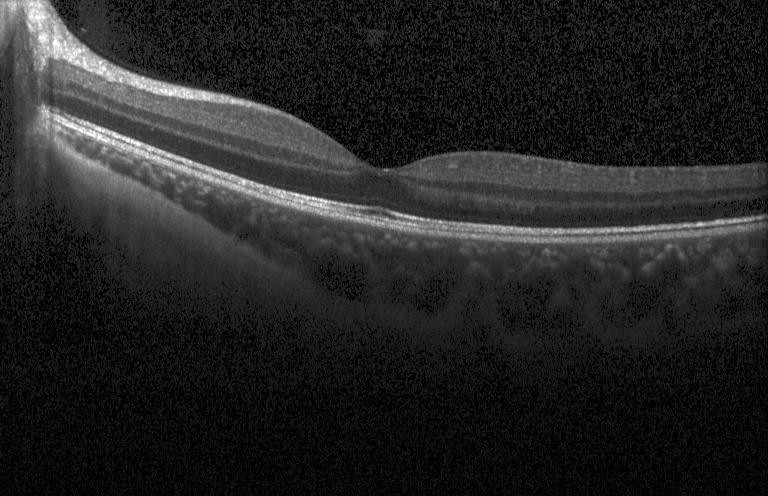

Dx: no choroidal neovascularization, no diabetic macular edema, and no drusen.